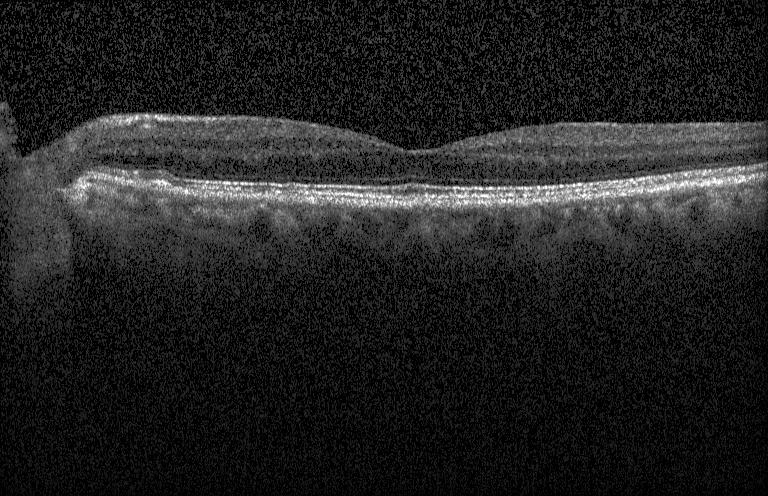

Impression: multiple drusen.